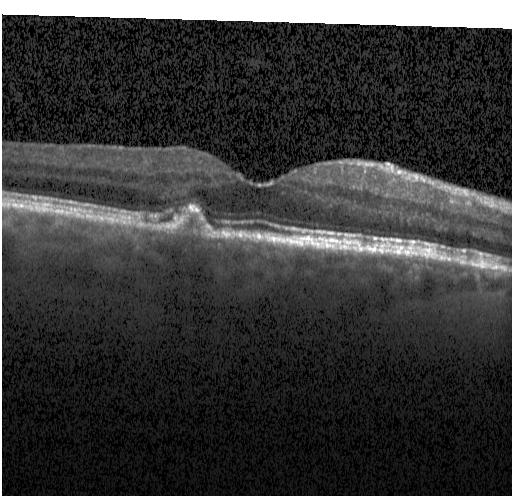 OCT B-scan — Impression: drusen.